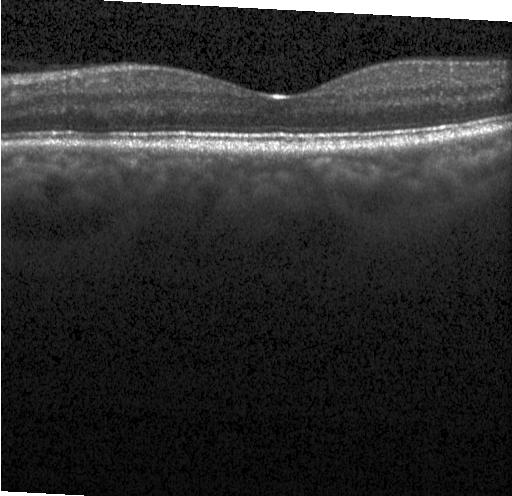

Heidelberg Spectralis OCT system; spectral-domain OCT; fovea-centered; optical coherence tomography B-scan — This B-scan demonstrates neither choroidal neovascularization, diabetic macular edema, nor drusen.